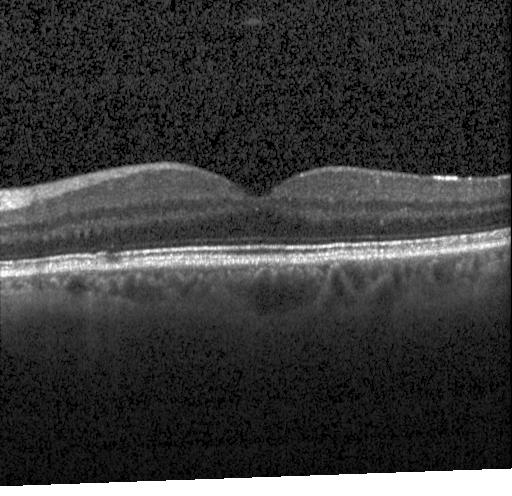

Optical coherence tomography scan. Acquired on a Heidelberg Spectralis. Spectral-domain OCT.
Macular OCT: neither choroidal neovascularization, diabetic macular edema, nor drusen.